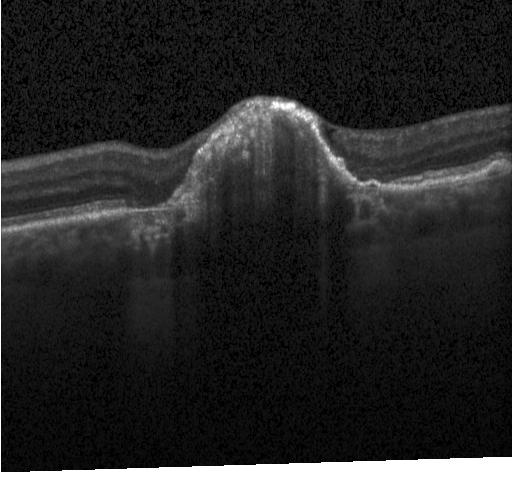

This B-scan demonstrates choroidal neovascularization.